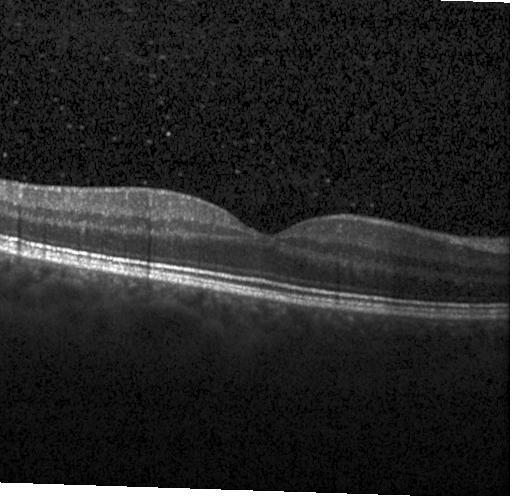

Optical coherence tomography B-scan. Spectral-domain optical coherence tomography — The scan shows no choroidal neovascularization, diabetic macular edema, or drusen.